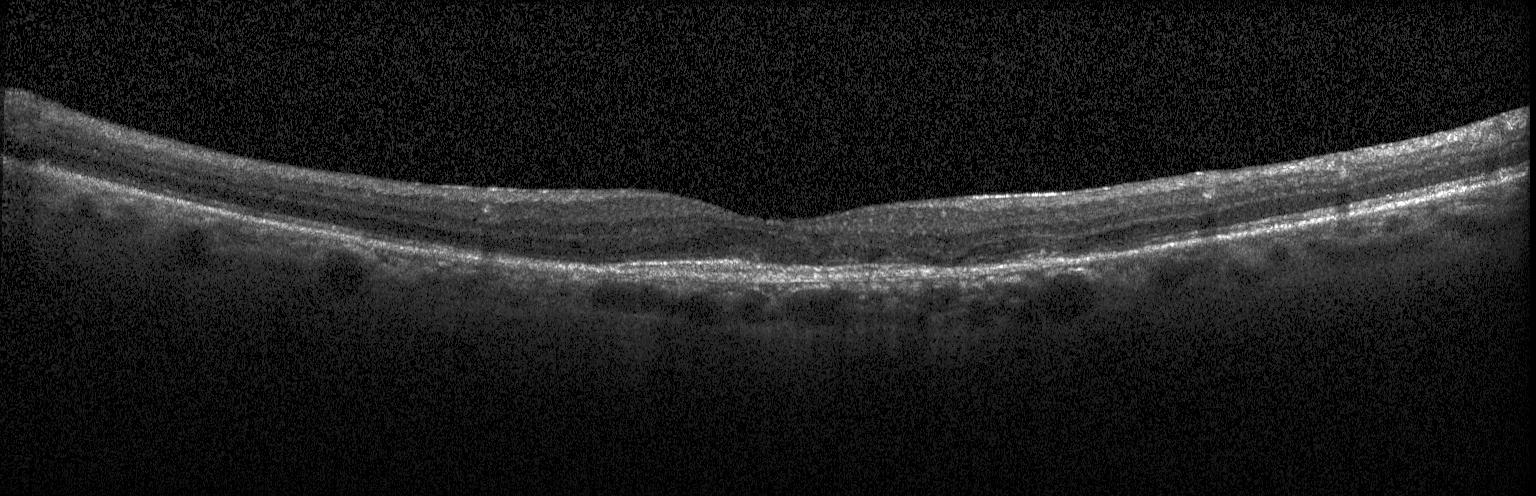 Retinal OCT B-scan
OCT finding: choroidal neovascularization.